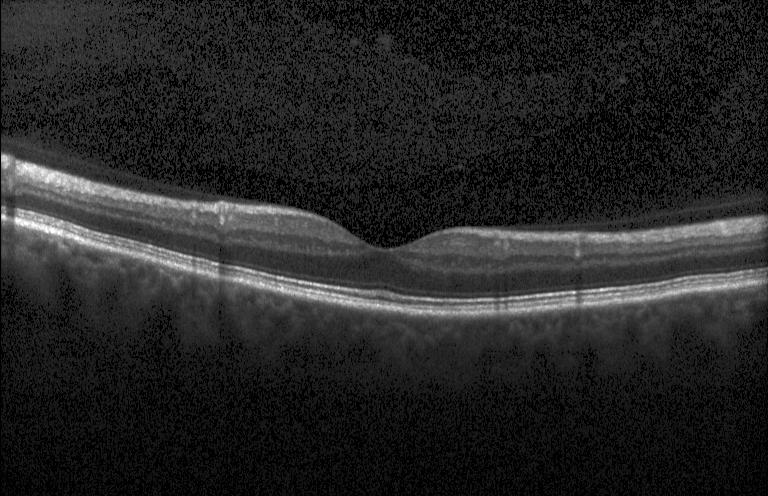

Acquired on a Heidelberg Spectralis; OCT line scan — The scan shows no choroidal neovascularization, diabetic macular edema, or drusen.